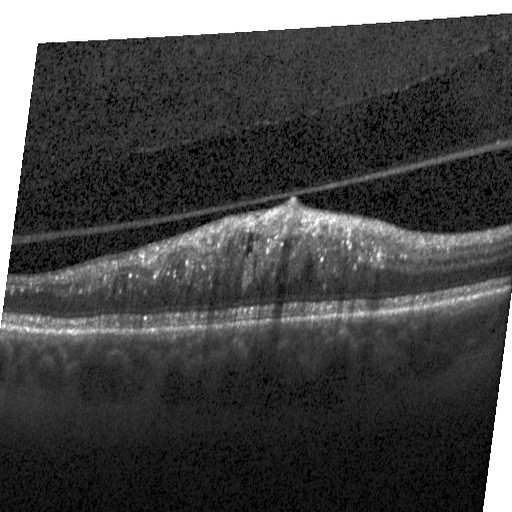 Optical coherence tomography scan. Heidelberg Spectralis. Macular OCT: diabetic macular edema (DME).